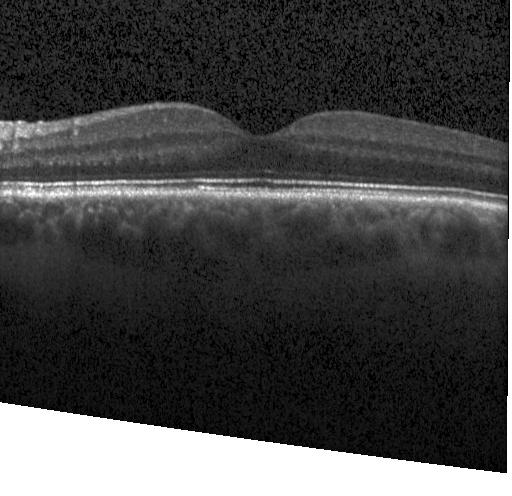
Optical coherence tomography B-scan, SD-OCT, fovea-centered, acquired on a Heidelberg Spectralis — Assessment: neither choroidal neovascularization, diabetic macular edema, nor drusen.